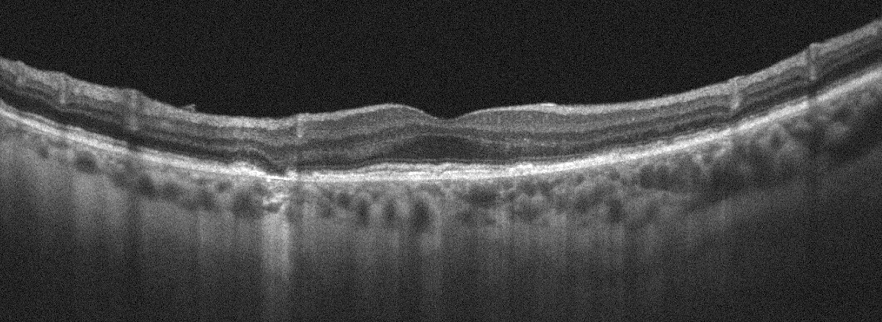

Optical coherence tomography B-scan.
Finding: age-related macular degeneration (AMD).